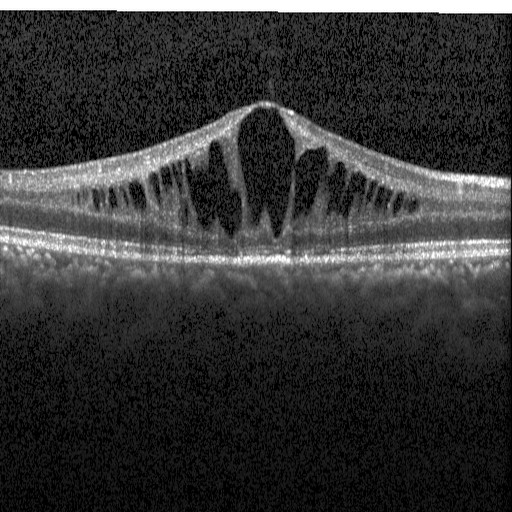
Macular OCT: diabetic macular edema.